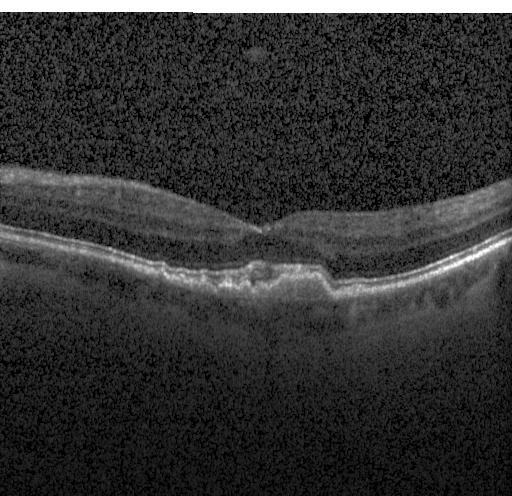
Macular OCT: drusen.